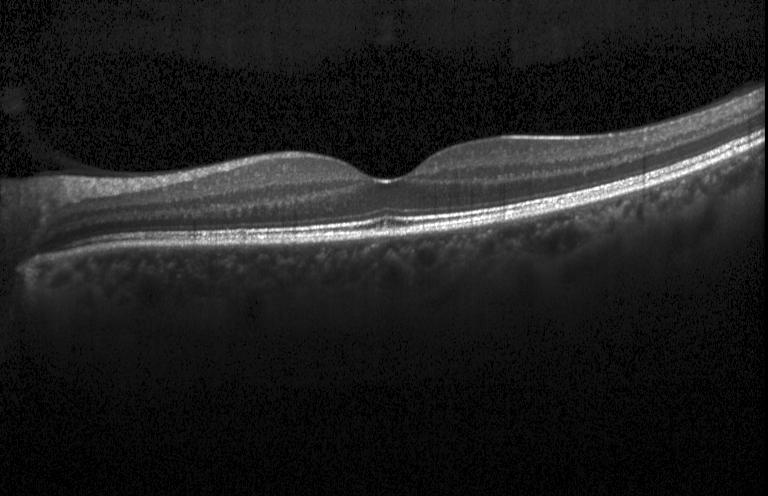
Macular scan. Retinal OCT B-scan. Spectral-domain OCT. Heidelberg Spectralis OCT system. Diagnosis: no choroidal neovascularization, diabetic macular edema, or drusen.